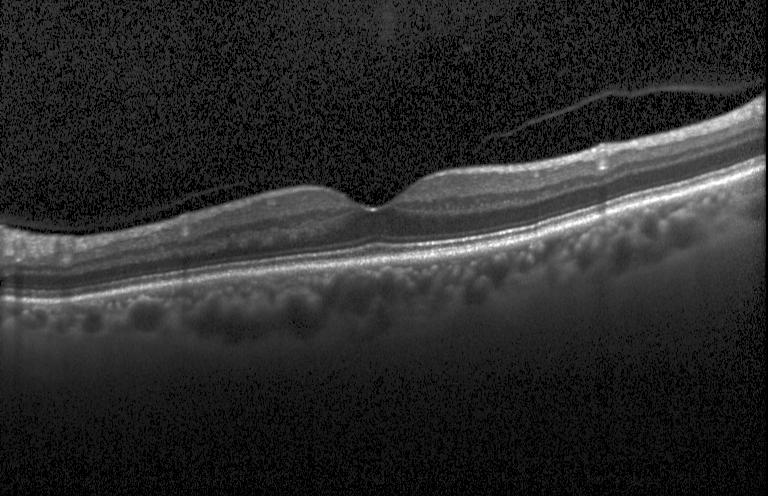

Impression: neither CNV, DME, nor drusen.